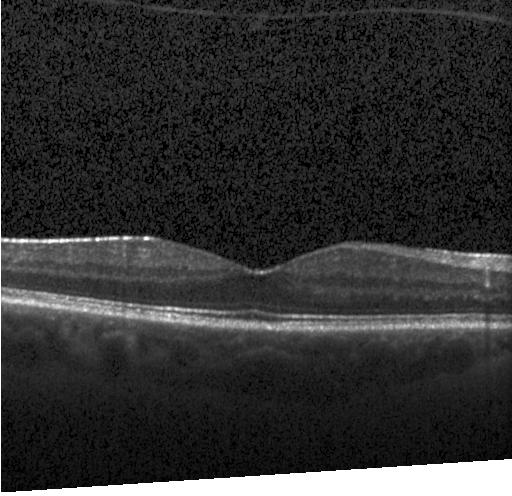 SD-OCT, optical coherence tomography B-scan, fovea-centered, Heidelberg Spectralis OCT system. Assessment: neither CNV, DME, nor drusen.